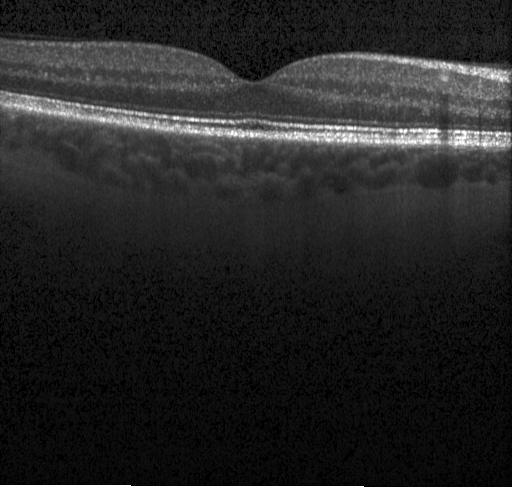 Instrument: Heidelberg Spectralis · spectral-domain OCT · optical coherence tomography B-scan · fovea-centered — OCT finding: neither choroidal neovascularization, diabetic macular edema, nor drusen.